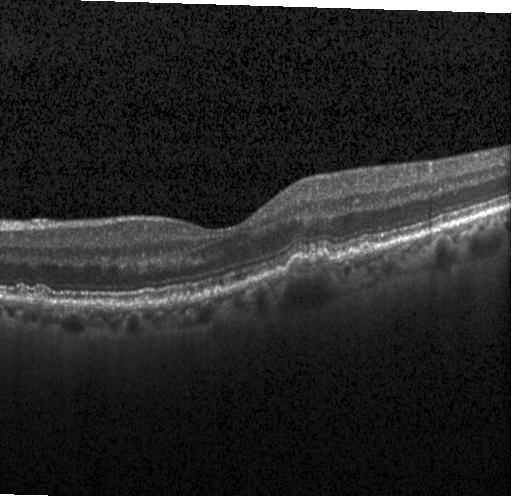

OCT line scan, instrument: Heidelberg Spectralis, SD-OCT, centered on the fovea.
Impression: multiple drusen.